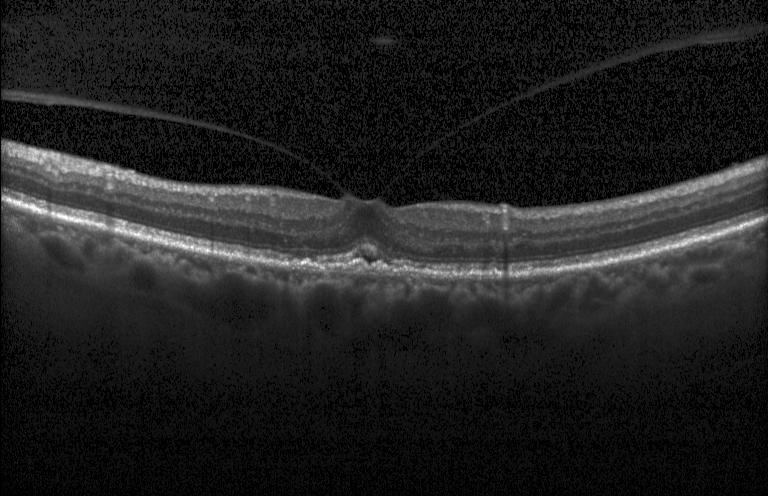
SD-OCT · acquired on a Heidelberg Spectralis · centered on the fovea · OCT B-scan — The scan shows a choroidal neovascular membrane.